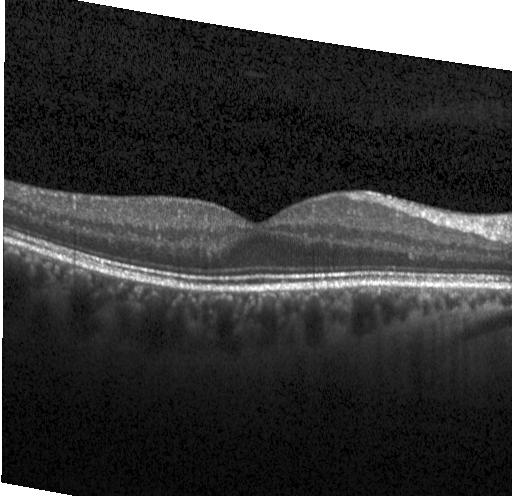

Macular OCT: no choroidal neovascularization, diabetic macular edema, or drusen.